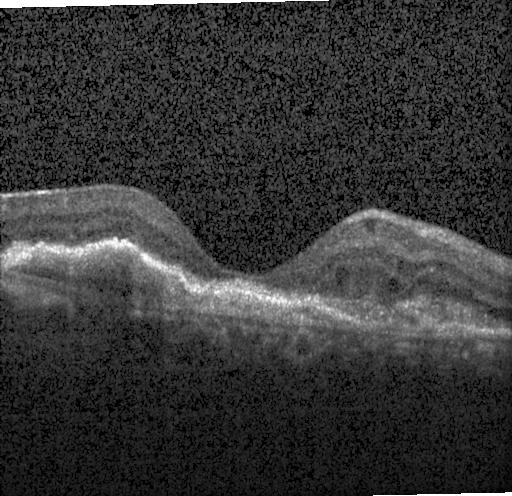
The scan shows a choroidal neovascular membrane.